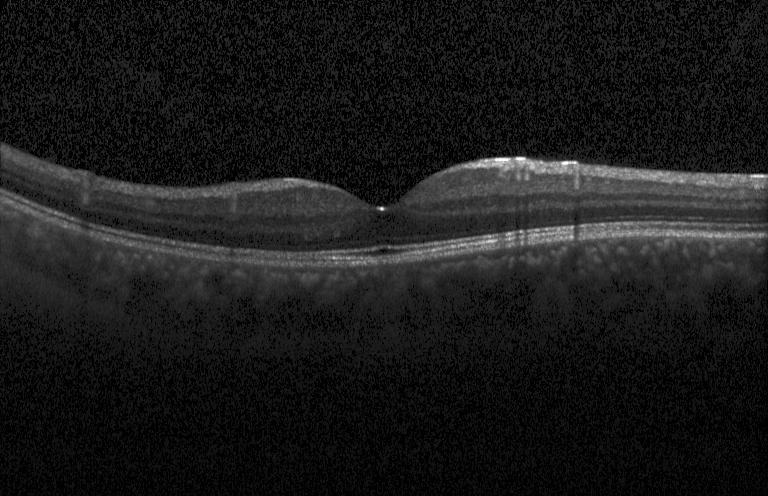 Macular OCT: no choroidal neovascularization, diabetic macular edema, or drusen.